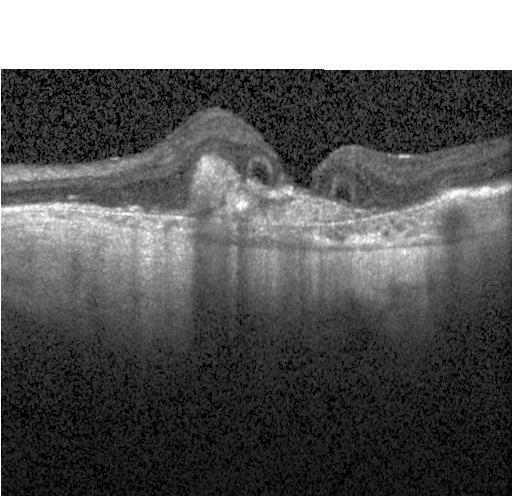
Retinal OCT cross-section
Diagnosis: a choroidal neovascular membrane.